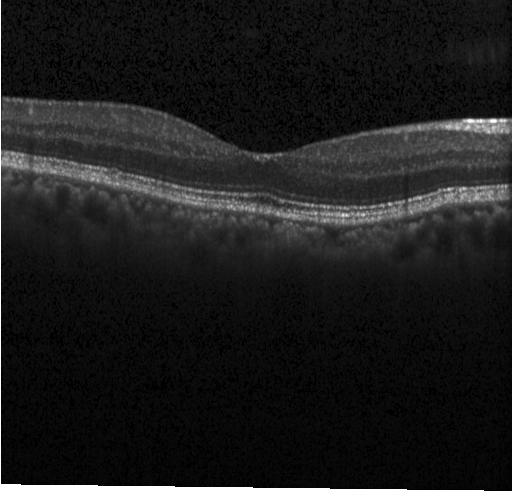 Dx: no choroidal neovascularization, diabetic macular edema, or drusen.